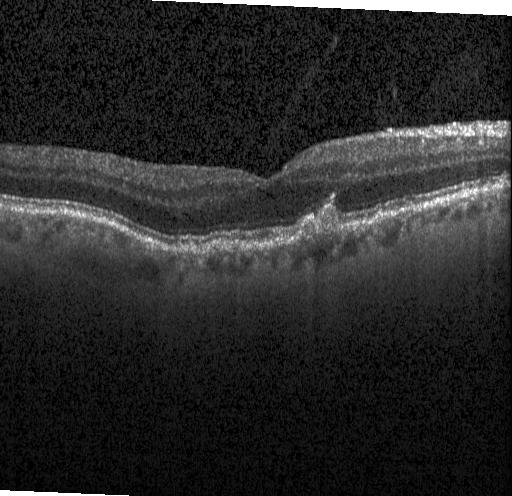
OCT line scan
Multiple drusen.